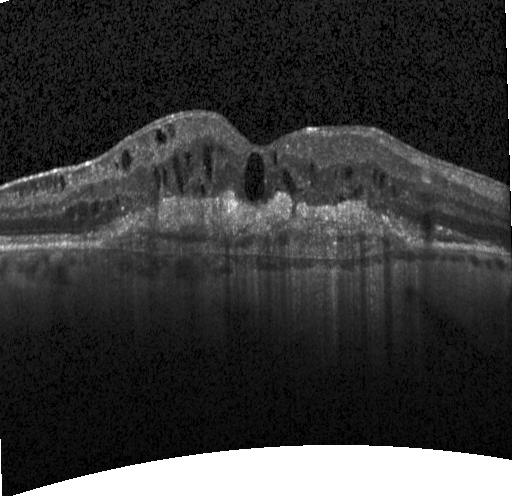
Macular OCT demonstrating a choroidal neovascular membrane.